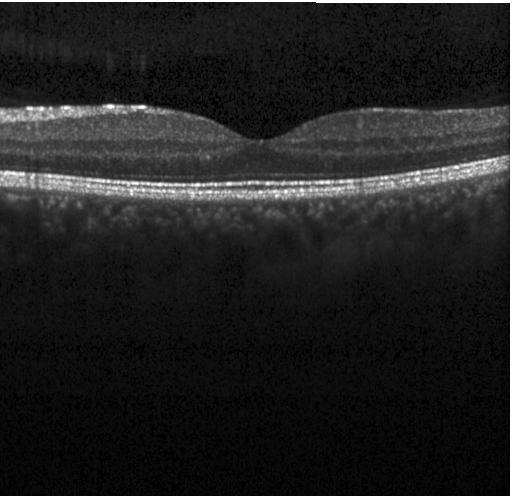

OCT line scan. This B-scan demonstrates neither choroidal neovascularization, diabetic macular edema, nor drusen.